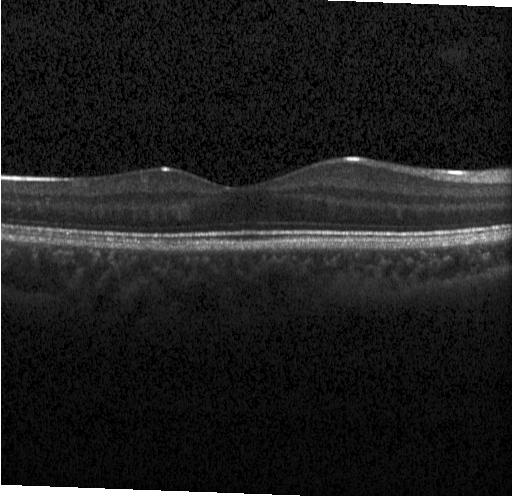

OCT line scan
Macular OCT: no choroidal neovascularization, no diabetic macular edema, and no drusen.